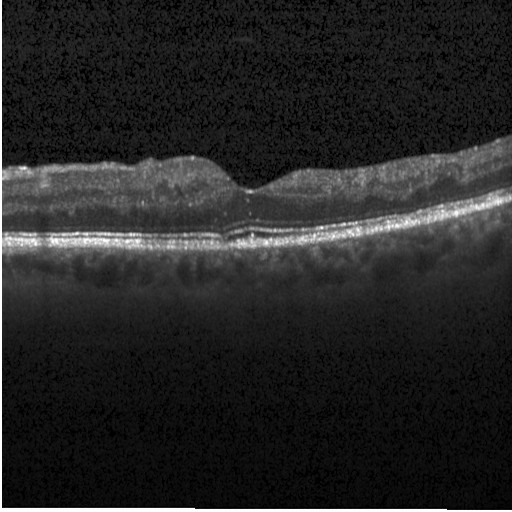
Dx: diabetic macular edema (DME).